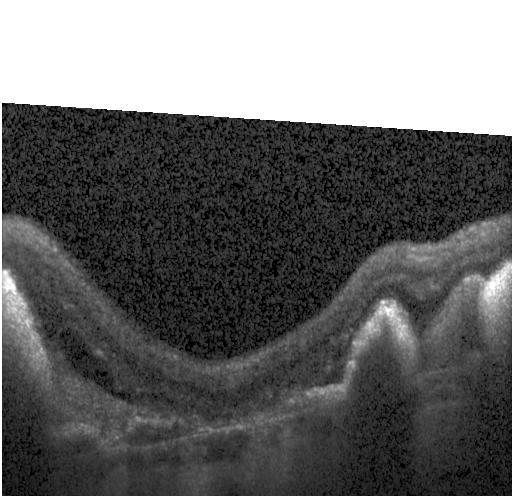
Macular OCT demonstrating a choroidal neovascular membrane.